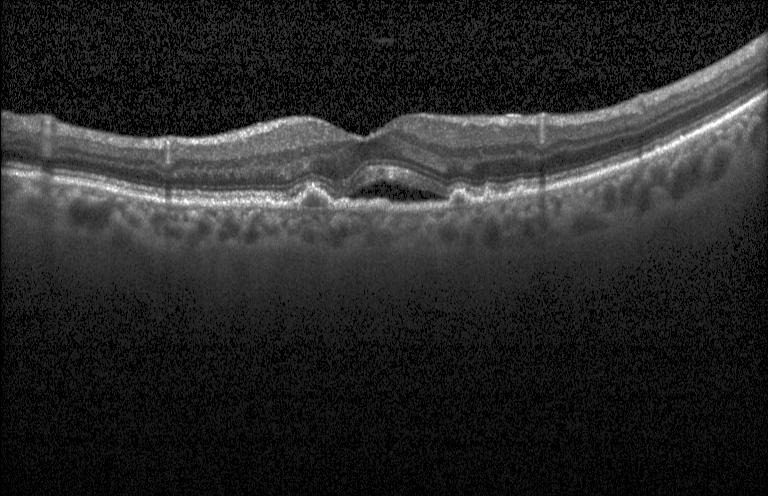

Optical coherence tomography scan. Horizontal scan through the fovea — Impression: a choroidal neovascular membrane.